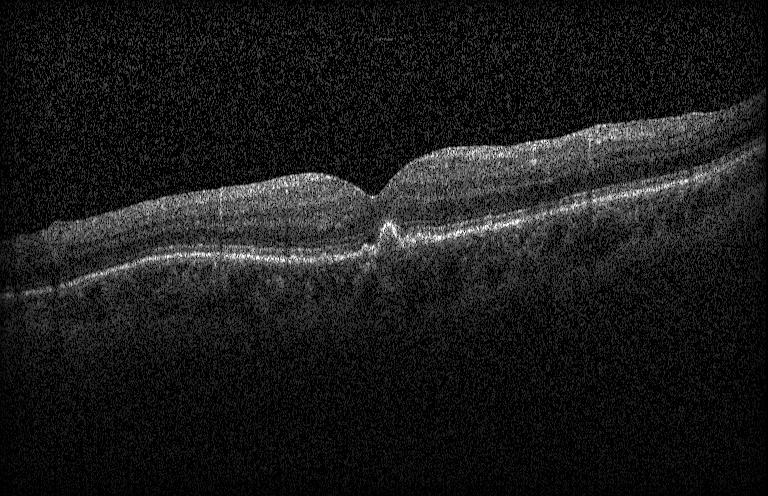

Diagnosis: drusen.